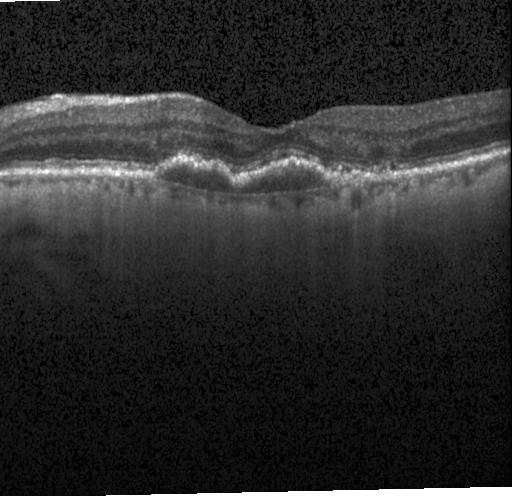

Retinal OCT cross-section showing CNV.